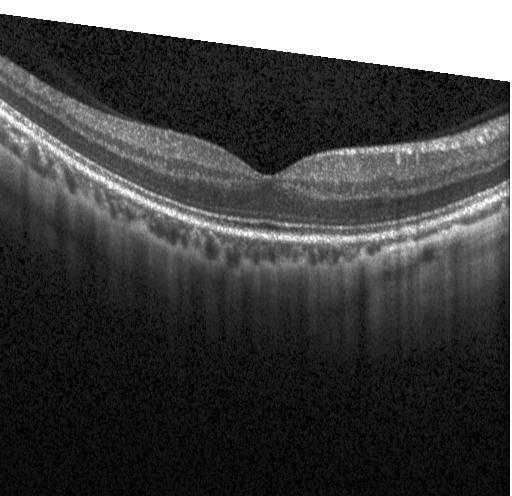

Finding: no choroidal neovascularization, no diabetic macular edema, and no drusen.